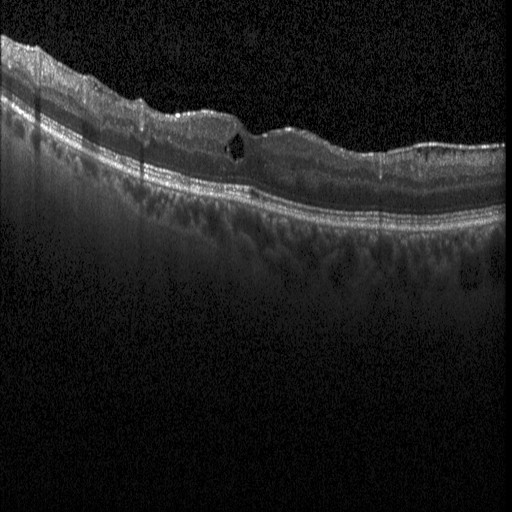
Optical coherence tomography scan. Spectral-domain OCT — Diabetic macular edema.